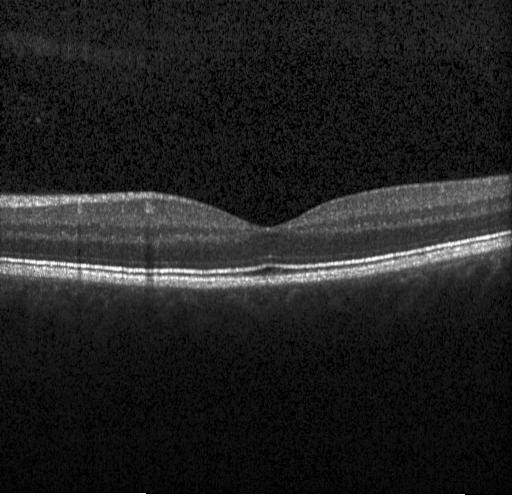

Finding: no choroidal neovascularization, diabetic macular edema, or drusen.